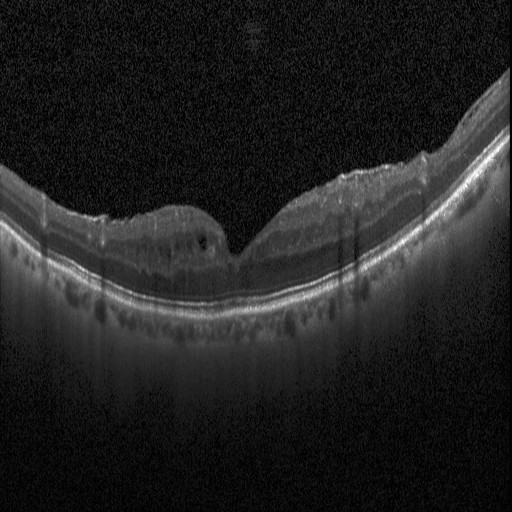
Impression: diabetic macular edema.